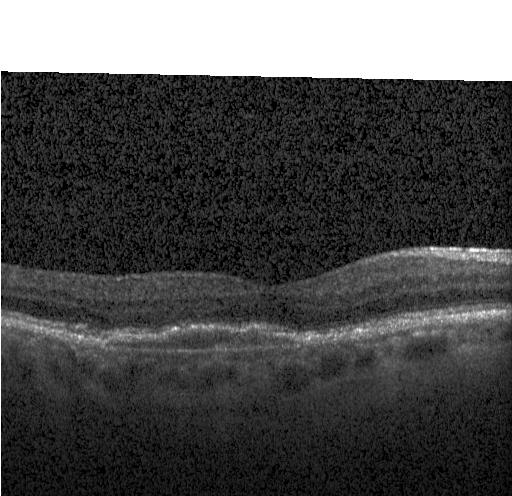

Retinal OCT cross-section; SD-OCT. Impression: choroidal neovascularization.